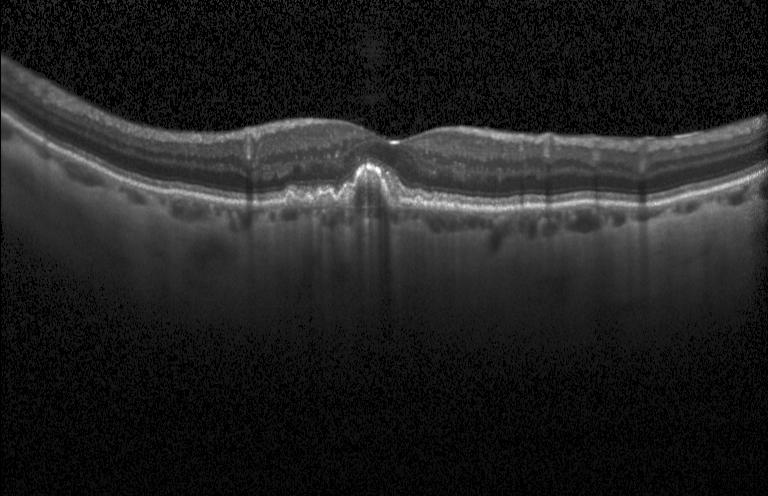 OCT B-scan showing drusen.